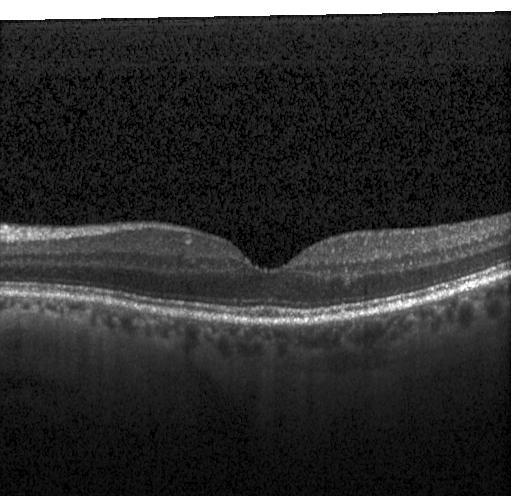

Optical coherence tomography B-scan.
Impression: neither CNV, DME, nor drusen.